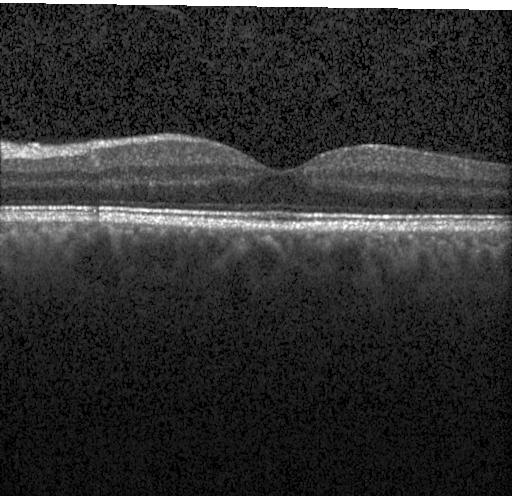 SD-OCT · retinal OCT B-scan.
The scan shows neither CNV, DME, nor drusen.